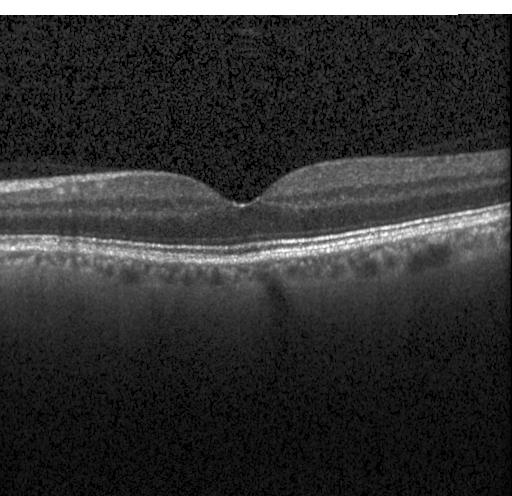
Diagnosis: no choroidal neovascularization, no diabetic macular edema, and no drusen.